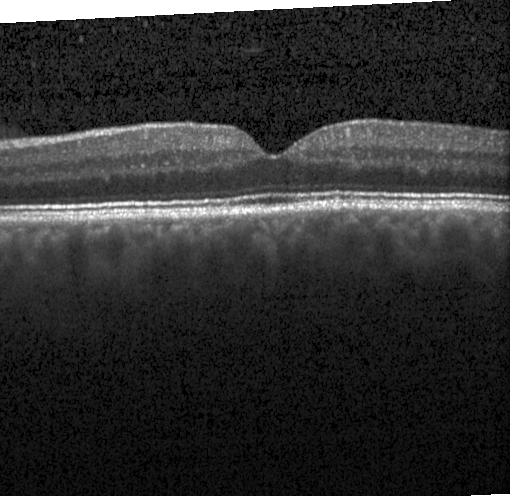
Optical coherence tomography scan.
Impression: no choroidal neovascularization, no diabetic macular edema, and no drusen.